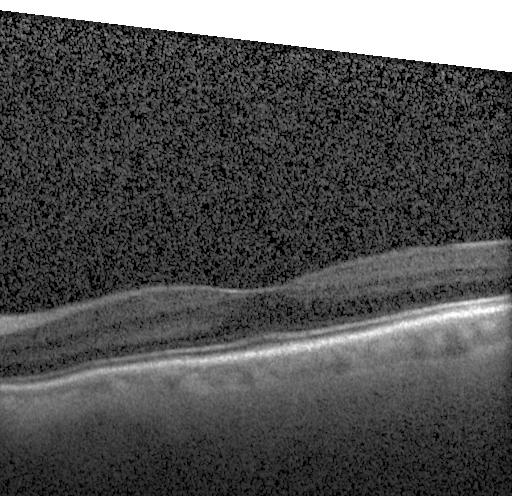
Macular OCT: no choroidal neovascularization, diabetic macular edema, or drusen.